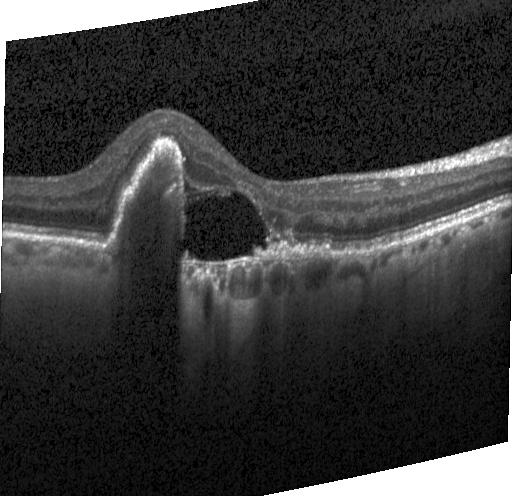 Acquired on a Heidelberg Spectralis, SD-OCT, retinal OCT cross-section, fovea-centered. Finding: a choroidal neovascular membrane.